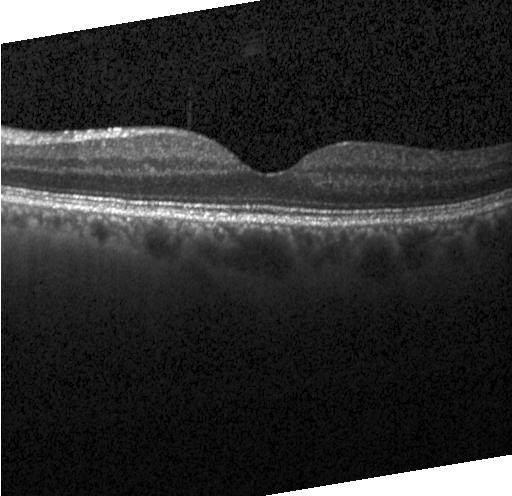
Impression: no evidence of choroidal neovascularization, diabetic macular edema, or drusen.